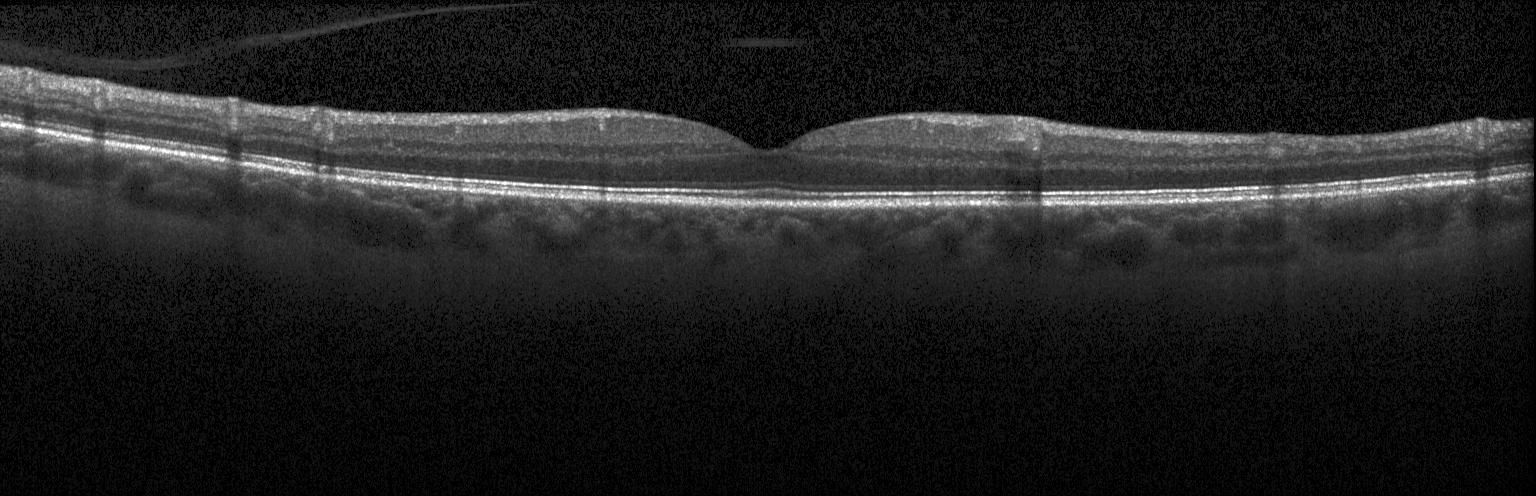 OCT finding: no choroidal neovascularization, diabetic macular edema, or drusen.